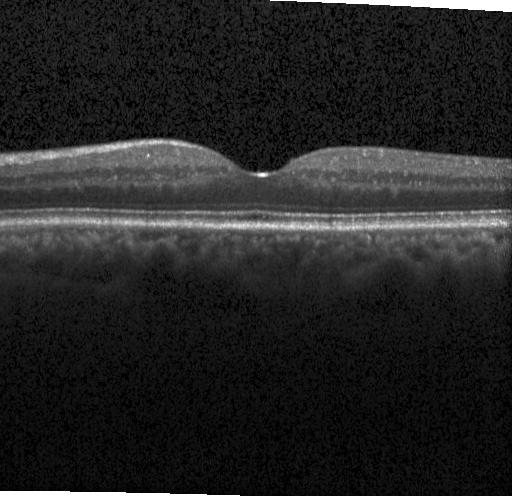

Retinal OCT cross-section.
Assessment: no choroidal neovascularization, no diabetic macular edema, and no drusen.